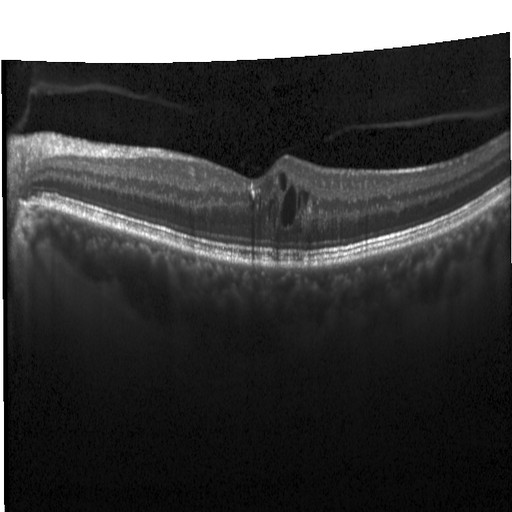 Spectral-domain optical coherence tomography · fovea-centered · optical coherence tomography scan
Diagnosis: DME.